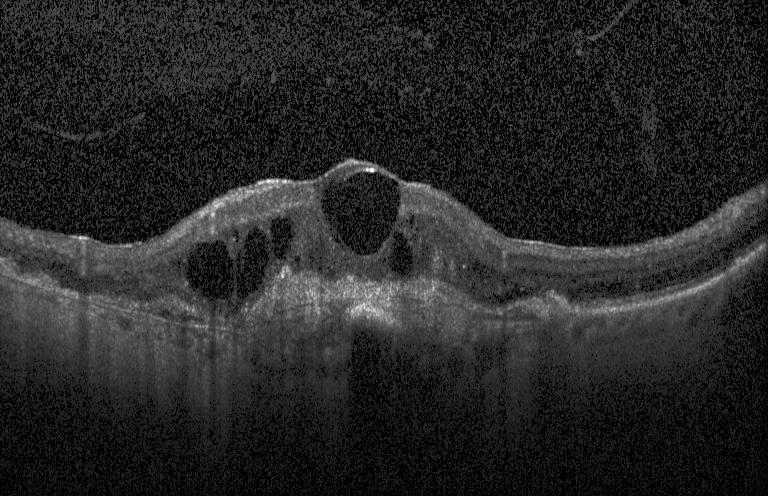

Retinal OCT cross-section showing a choroidal neovascular membrane.